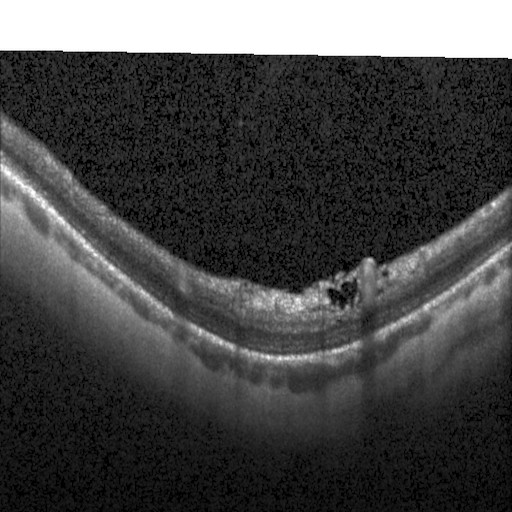
OCT line scan · Heidelberg Spectralis.
The scan shows diabetic macular edema.